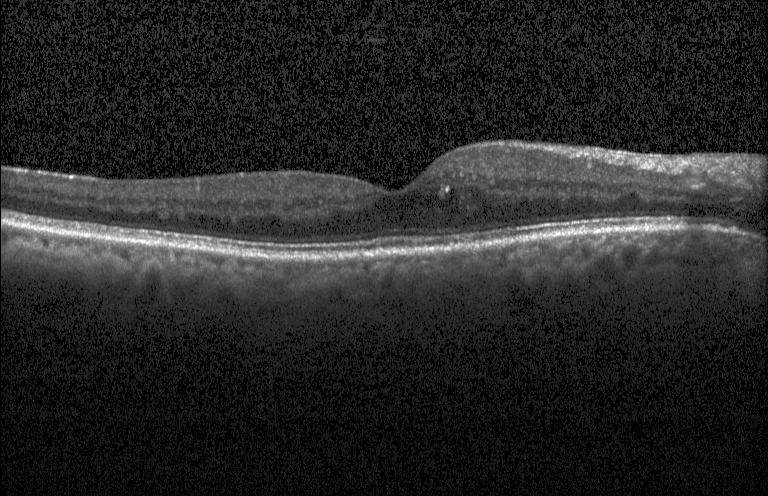

The scan shows diabetic macular edema (DME).